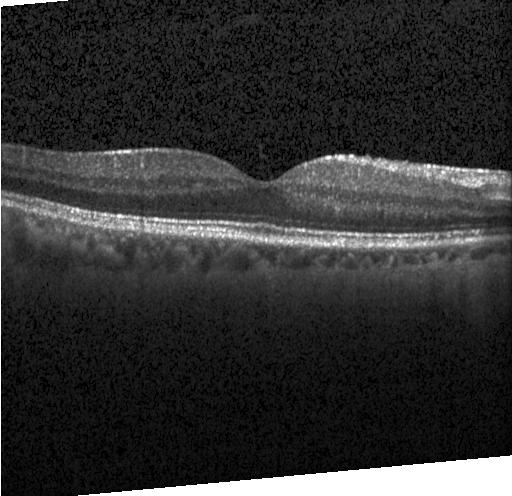

Macular OCT: no CNV, DME, or drusen.